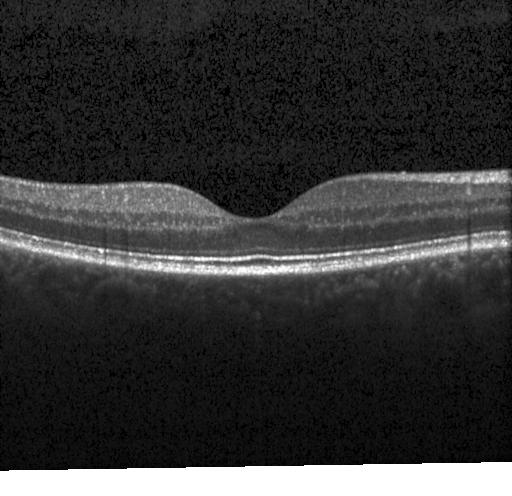 OCT line scan. SD-OCT. Through the macula. Diagnosis: no CNV, DME, or drusen.